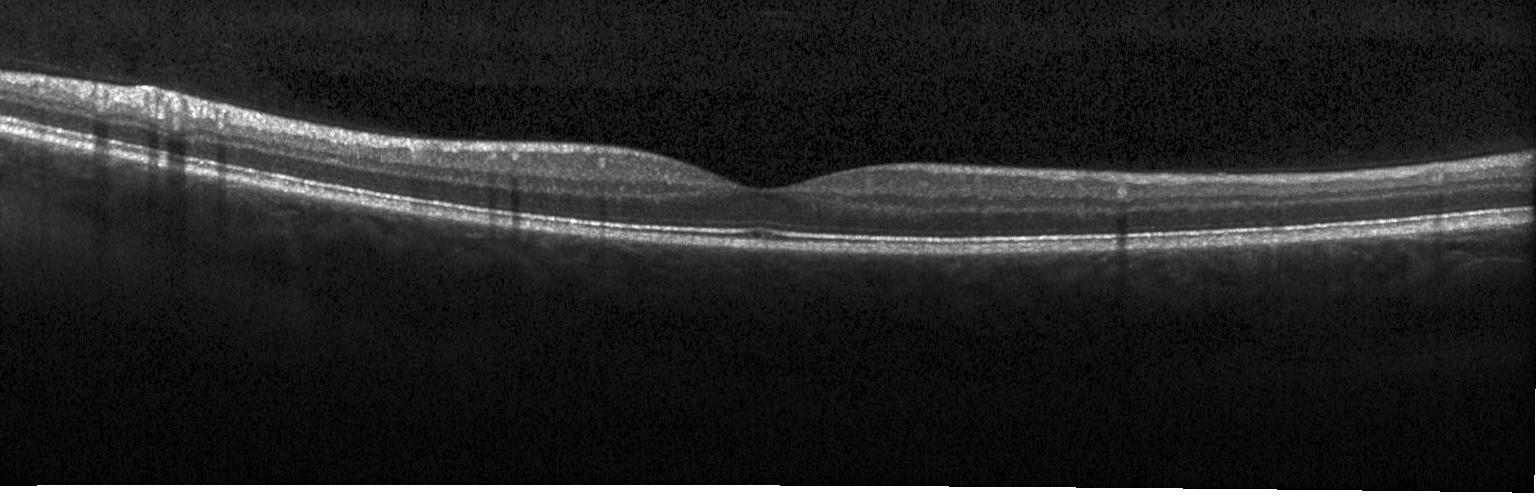

Optical coherence tomography B-scan — Finding: no choroidal neovascularization, no diabetic macular edema, and no drusen.